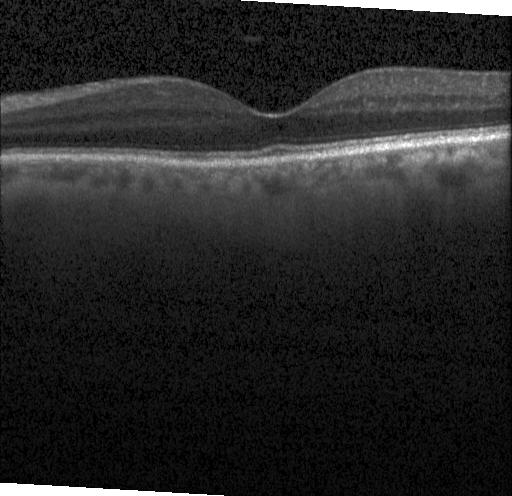
Centered on the fovea. Spectral-domain OCT. Heidelberg Spectralis OCT system. Optical coherence tomography B-scan — The scan shows no evidence of choroidal neovascularization, diabetic macular edema, or drusen.